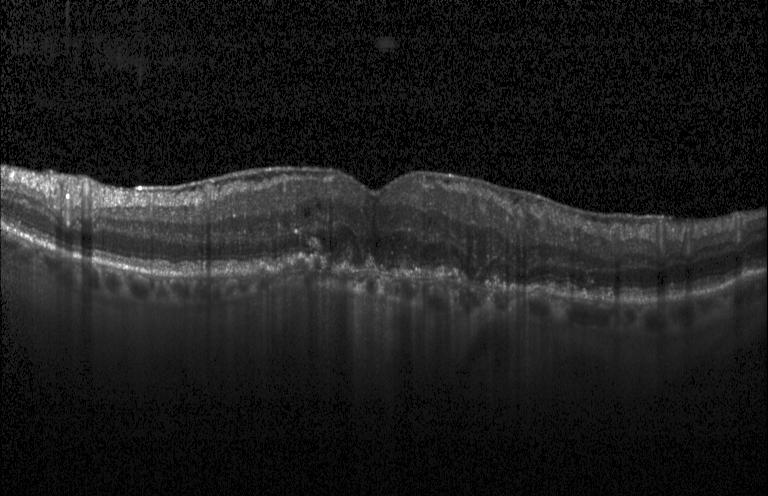

This B-scan demonstrates choroidal neovascularization (CNV).